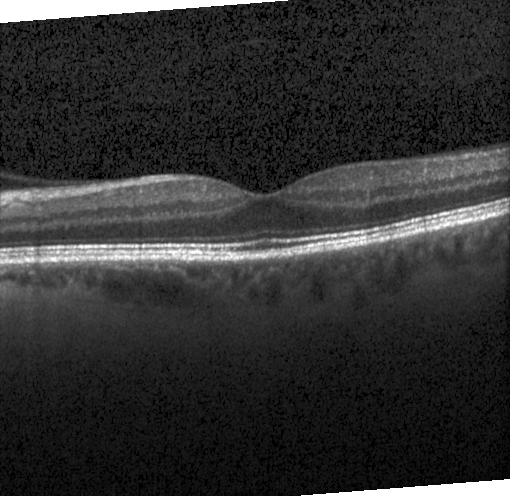
OCT B-scan. Acquired on a Heidelberg Spectralis.
Assessment: no evidence of choroidal neovascularization, diabetic macular edema, or drusen.